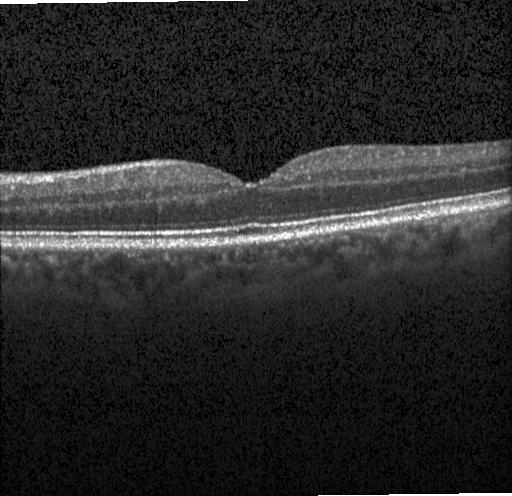
Spectral-domain optical coherence tomography, Heidelberg Spectralis, retinal OCT B-scan
Assessment: neither choroidal neovascularization, diabetic macular edema, nor drusen.